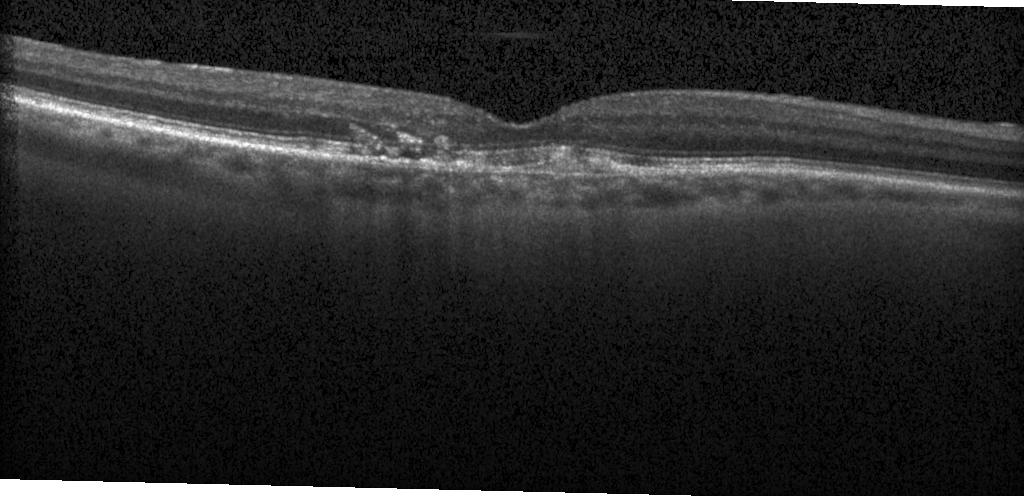

Macular OCT demonstrating a choroidal neovascular membrane.